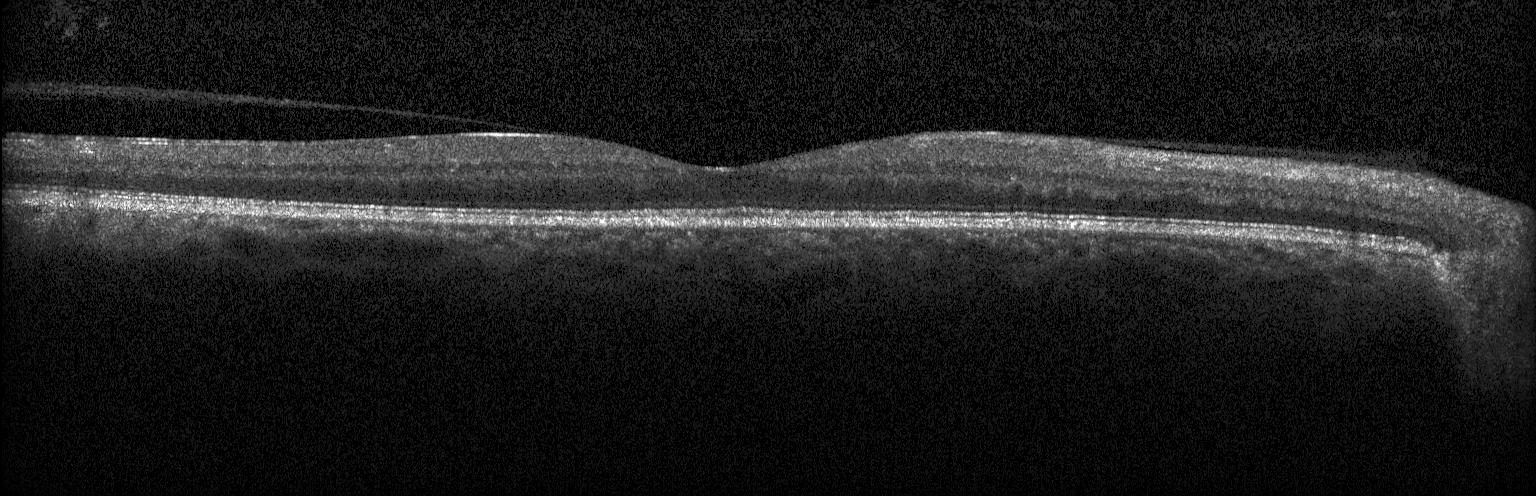
Through the macula; Heidelberg Spectralis OCT system; retinal OCT B-scan
Diagnosis: no choroidal neovascularization, no diabetic macular edema, and no drusen.